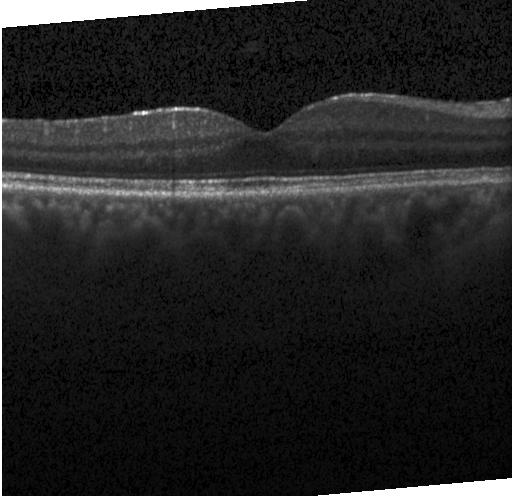

Macular OCT: neither choroidal neovascularization, diabetic macular edema, nor drusen.